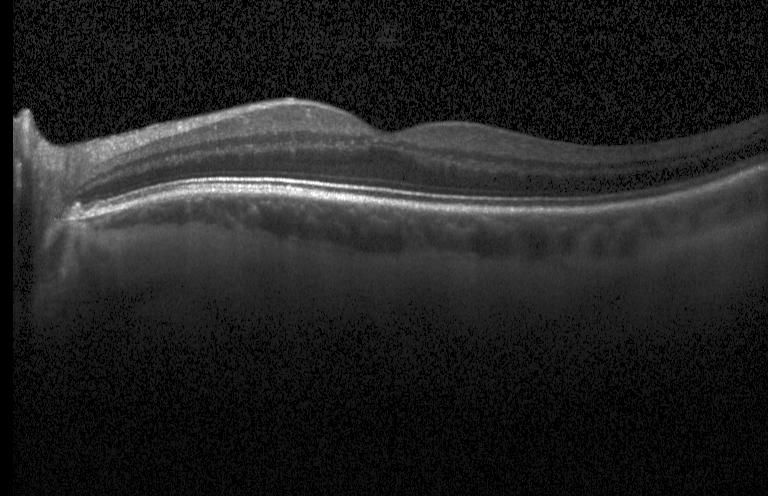
Macular OCT: no evidence of CNV, DME, or drusen.